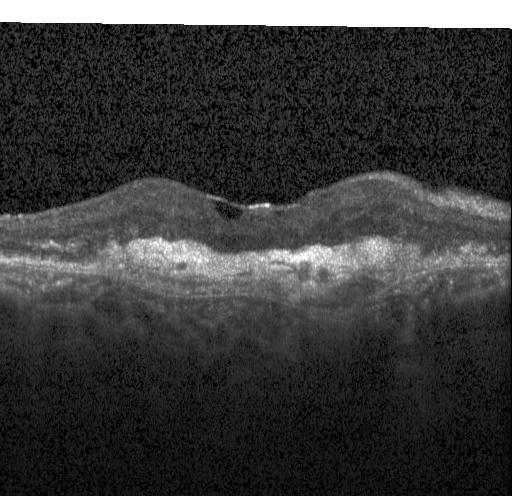
Finding: choroidal neovascularization.